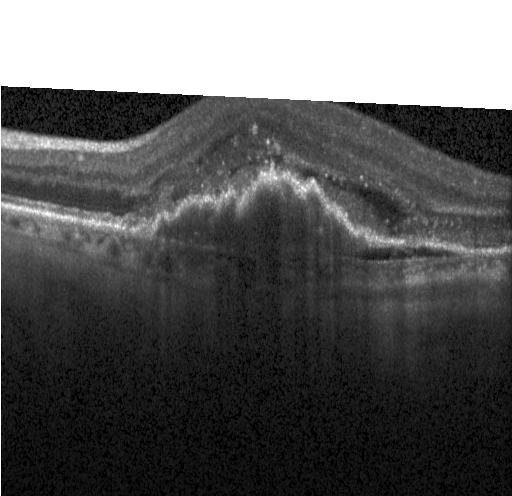 Spectral-domain OCT B-scan: choroidal neovascularization (CNV).